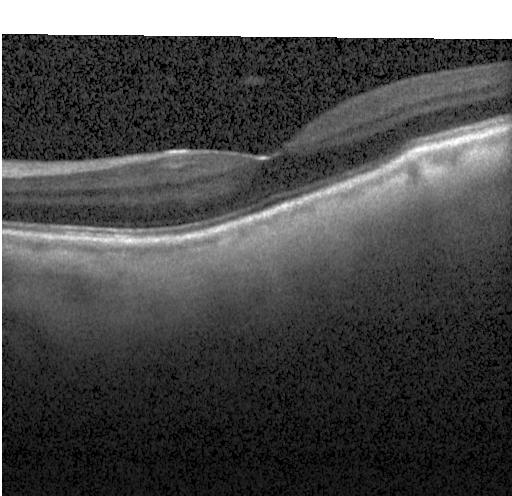 OCT scan showing neither choroidal neovascularization, diabetic macular edema, nor drusen.